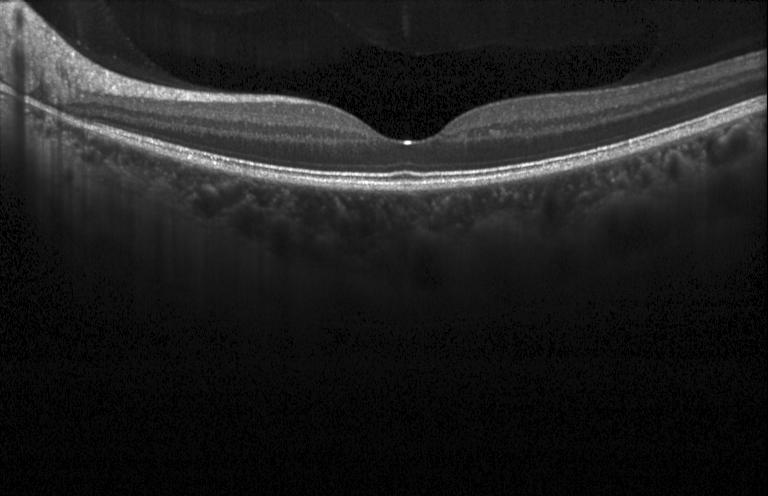 Acquired on a Heidelberg Spectralis. Spectral-domain OCT. Optical coherence tomography B-scan. Assessment: neither choroidal neovascularization, diabetic macular edema, nor drusen.